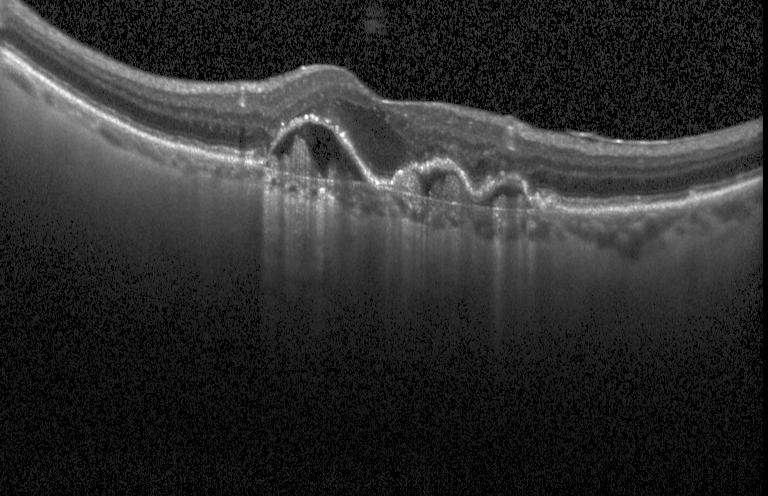 Finding: choroidal neovascularization (CNV).